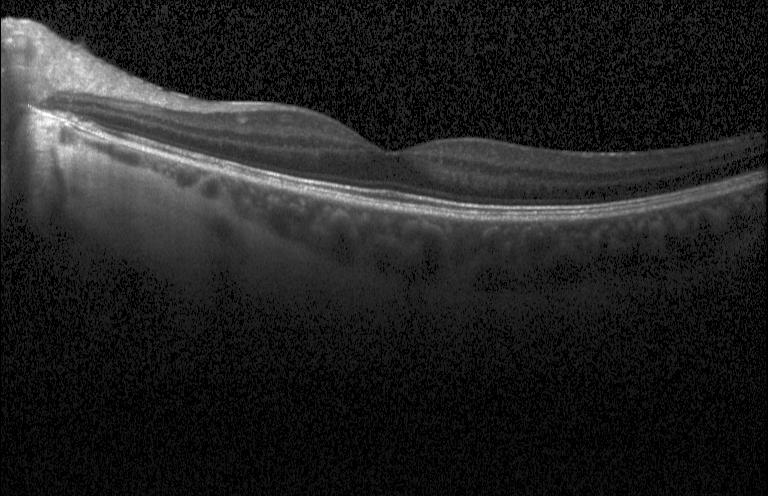 The scan shows neither CNV, DME, nor drusen.